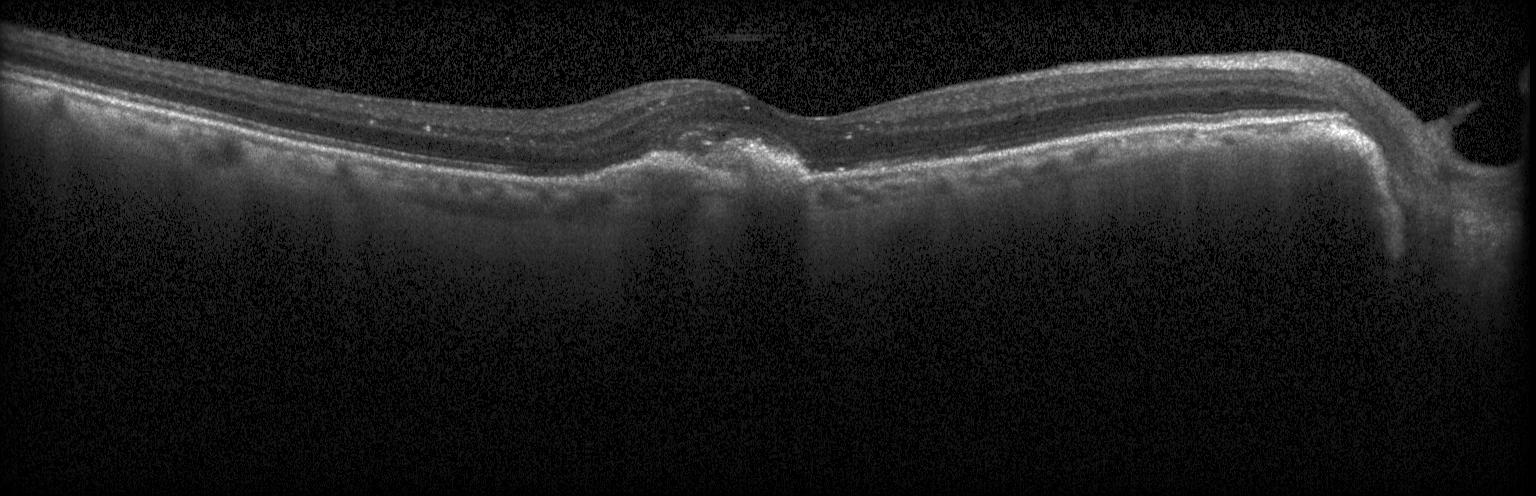
Heidelberg Spectralis OCT system · spectral-domain OCT · optical coherence tomography scan · through the macula. Impression: a choroidal neovascular membrane.